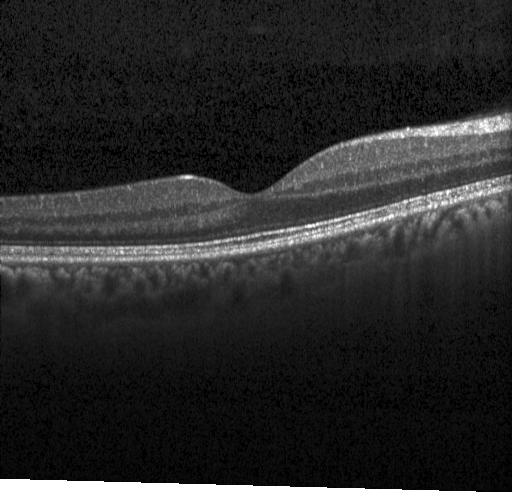
Horizontal scan through the fovea · optical coherence tomography scan.
Impression: no choroidal neovascularization, diabetic macular edema, or drusen.